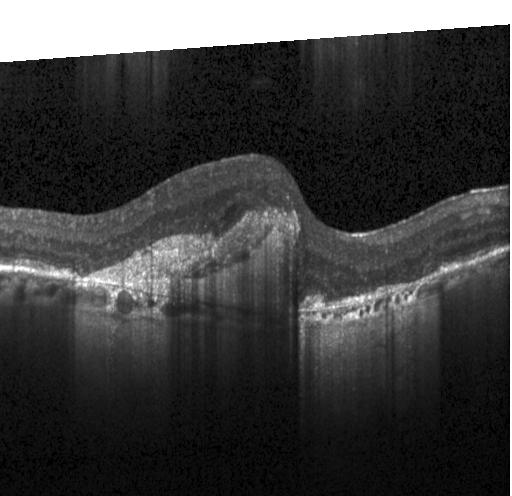
Macular scan · Heidelberg Spectralis · OCT B-scan · spectral-domain OCT — Impression: a choroidal neovascular membrane.